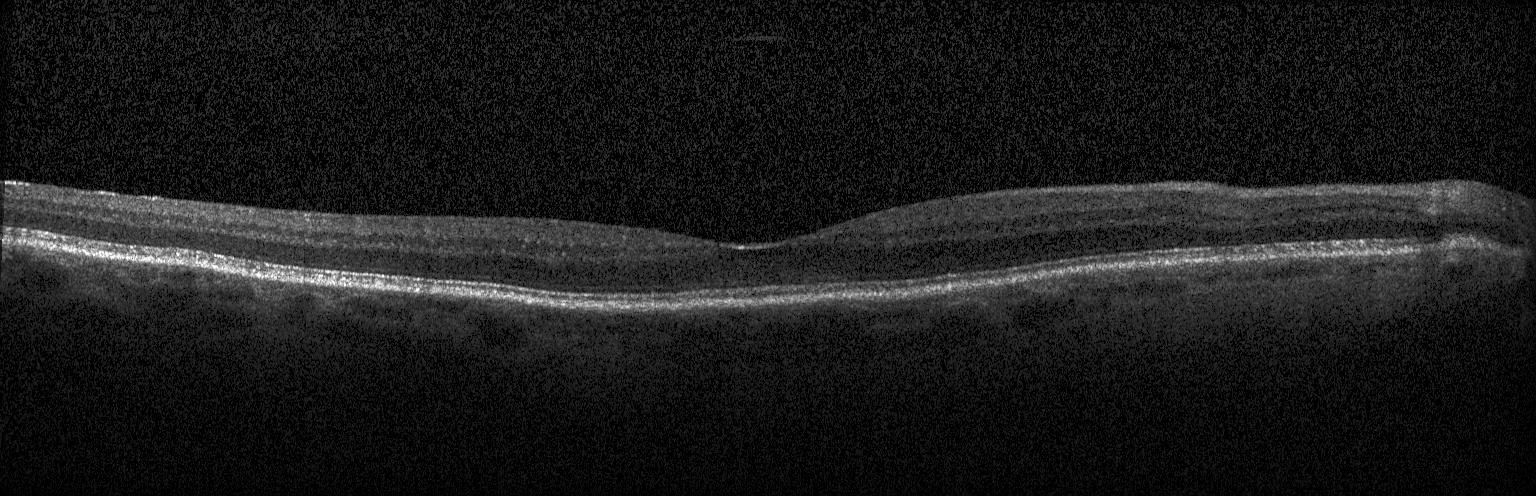
Heidelberg Spectralis. Spectral-domain OCT. Retinal OCT B-scan. Horizontal scan through the fovea
The scan shows neither CNV, DME, nor drusen.